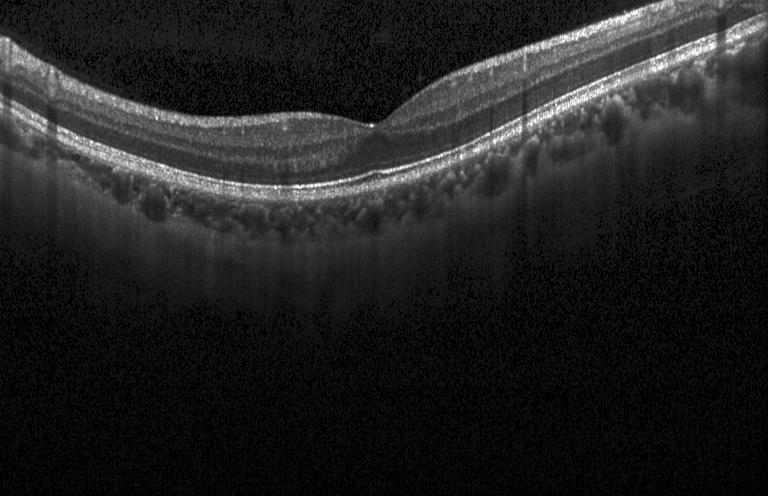

Retinal OCT B-scan · through the macula · spectral-domain OCT · Heidelberg Spectralis. Assessment: no evidence of CNV, DME, or drusen.